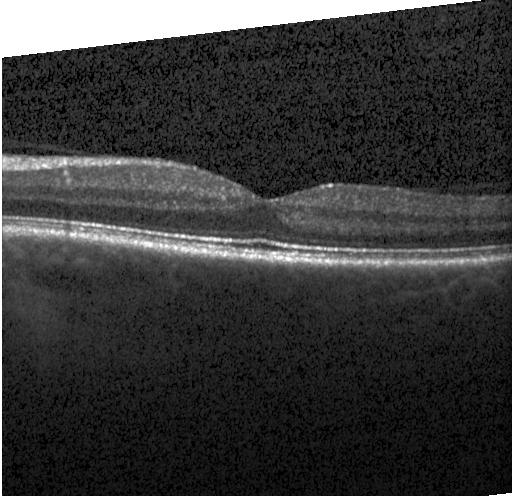
OCT scan showing no CNV, no DME, and no drusen.